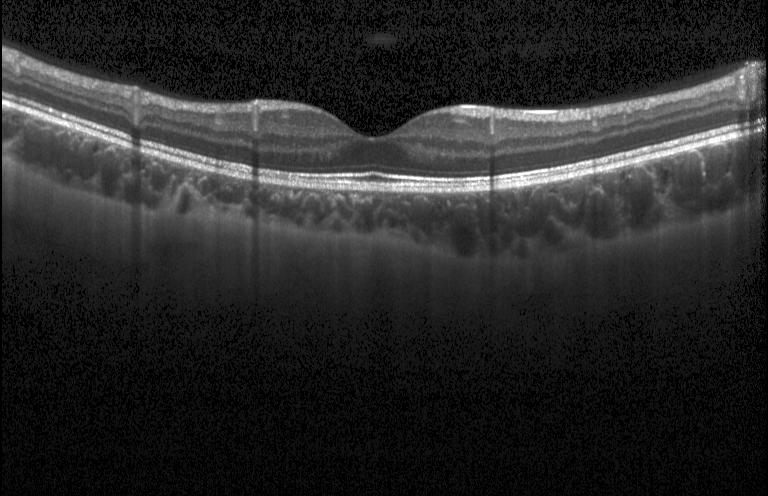

Dx: no choroidal neovascularization, diabetic macular edema, or drusen.